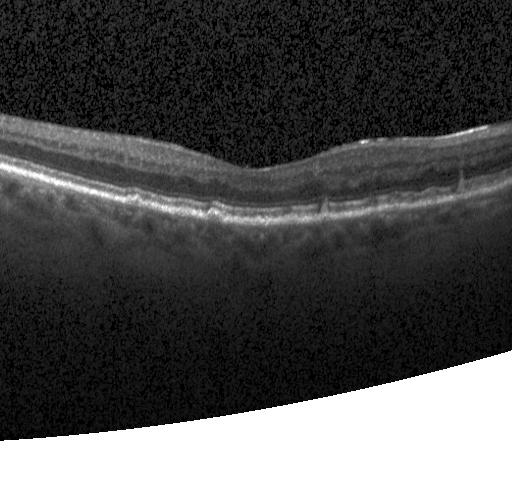
Finding: multiple drusen.